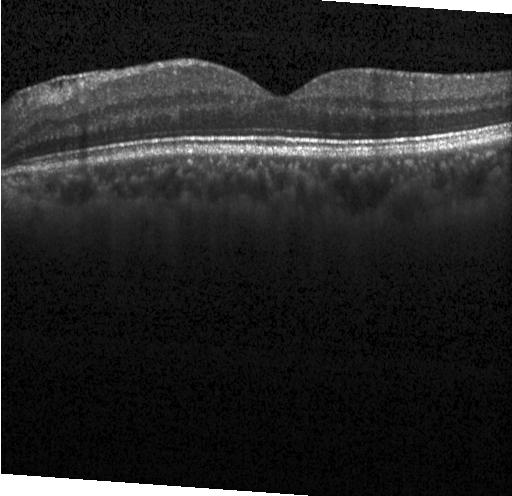

OCT line scan. Diagnosis: no choroidal neovascularization, diabetic macular edema, or drusen.